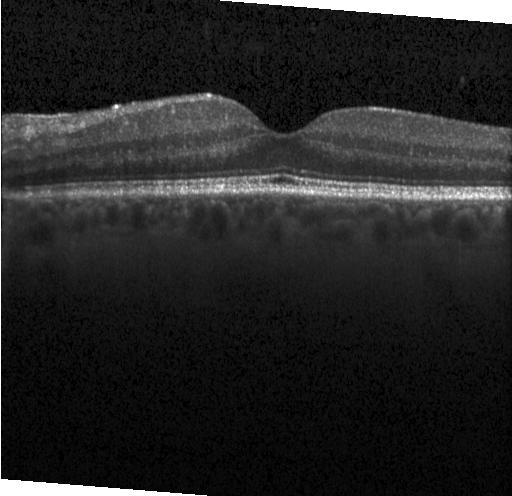 Heidelberg Spectralis. OCT line scan. Horizontal scan through the fovea — Diagnosis: no CNV, no DME, and no drusen.